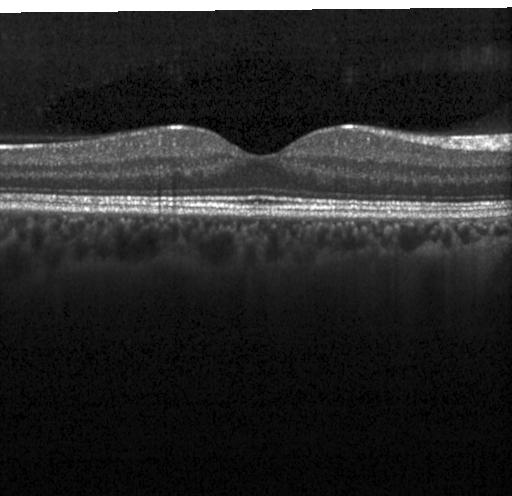 Retinal OCT cross-section
Diagnosis: neither CNV, DME, nor drusen.